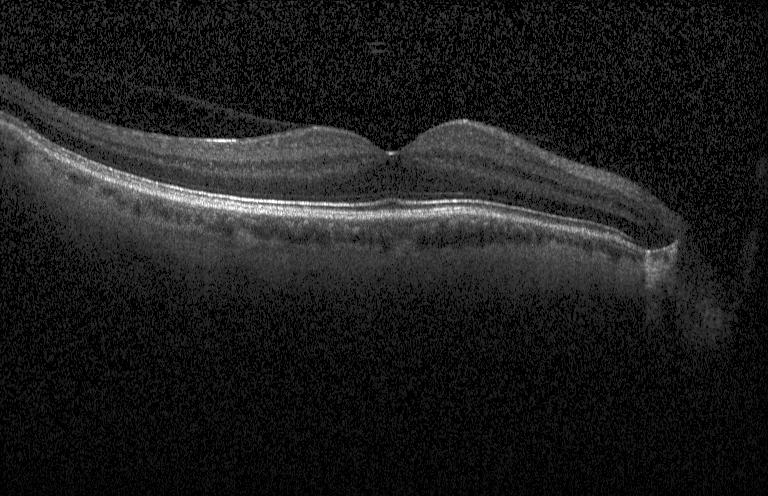

OCT finding: no evidence of CNV, DME, or drusen.